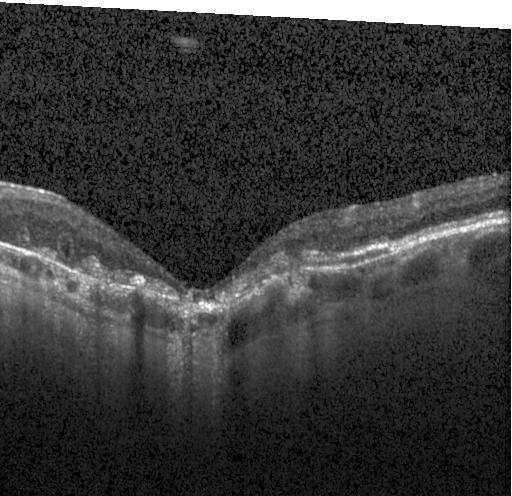

Optical coherence tomography scan. This B-scan demonstrates a choroidal neovascular membrane.